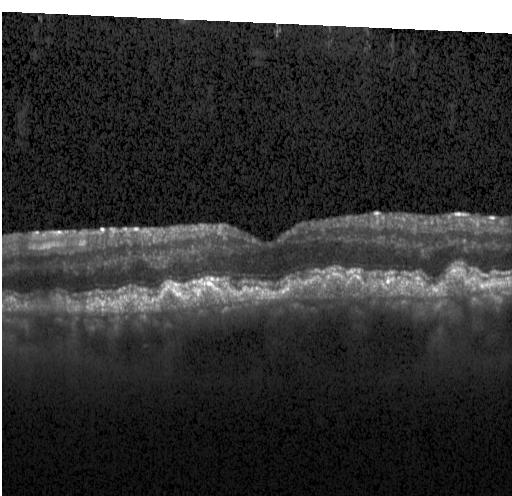
OCT scan showing choroidal neovascularization (CNV).